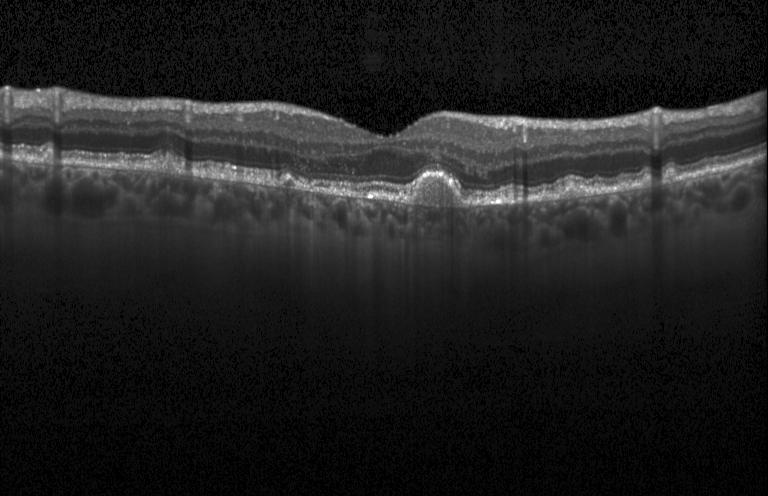
Spectral-domain OCT; acquired on a Heidelberg Spectralis; optical coherence tomography B-scan.
Diagnosis: drusen.